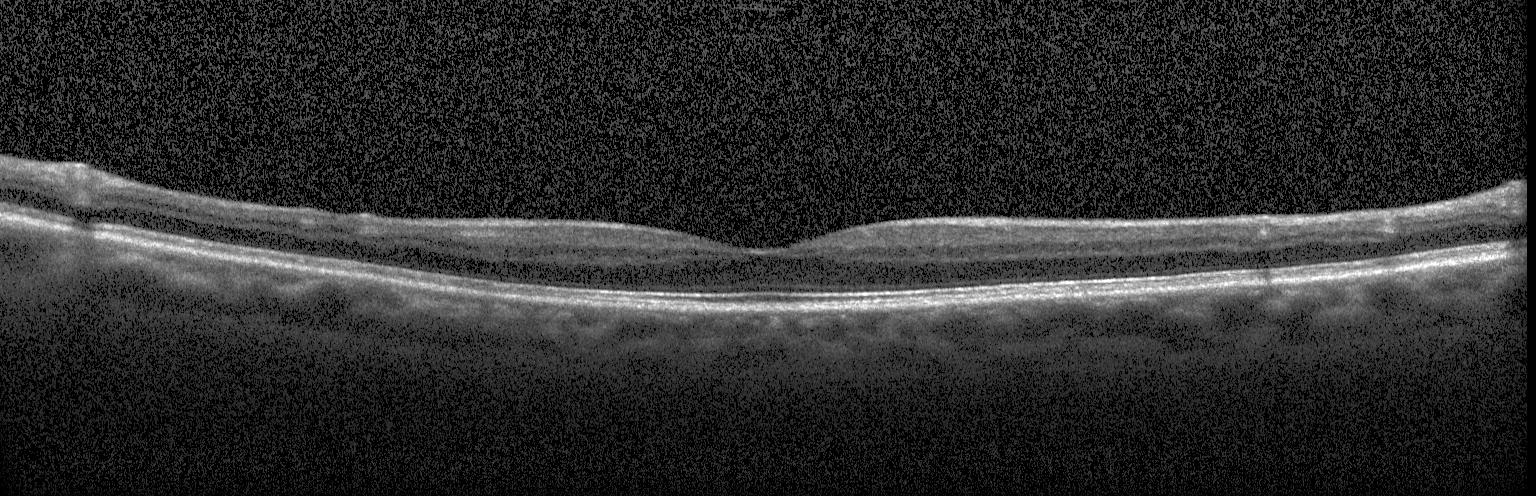

Dx: no choroidal neovascularization, diabetic macular edema, or drusen.